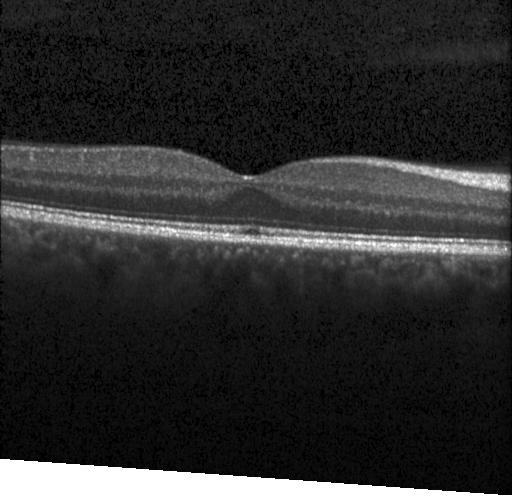
Optical coherence tomography scan · Heidelberg Spectralis OCT system
Finding: neither choroidal neovascularization, diabetic macular edema, nor drusen.